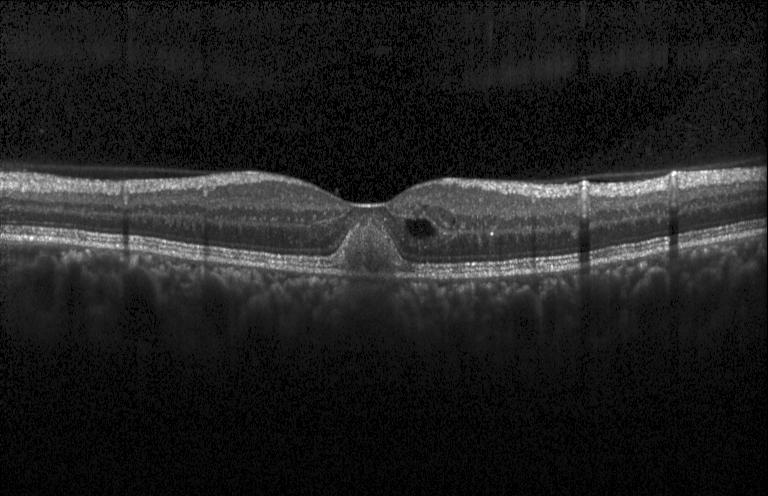
Macular OCT: a choroidal neovascular membrane.